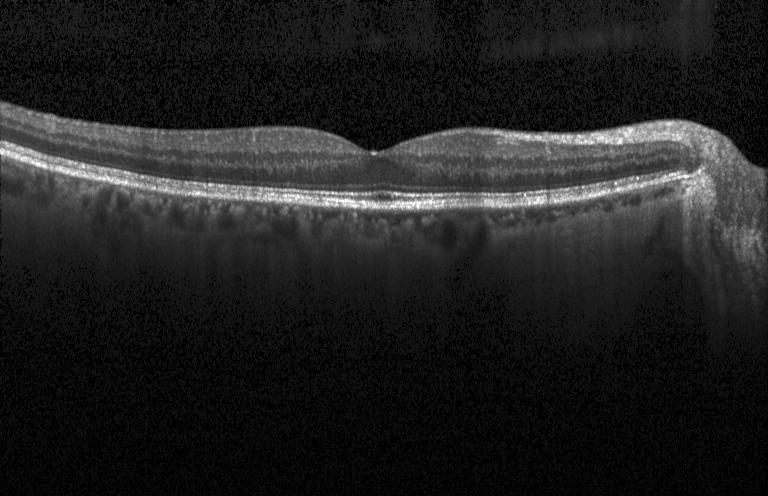

OCT B-scan. Finding: no choroidal neovascularization, diabetic macular edema, or drusen.